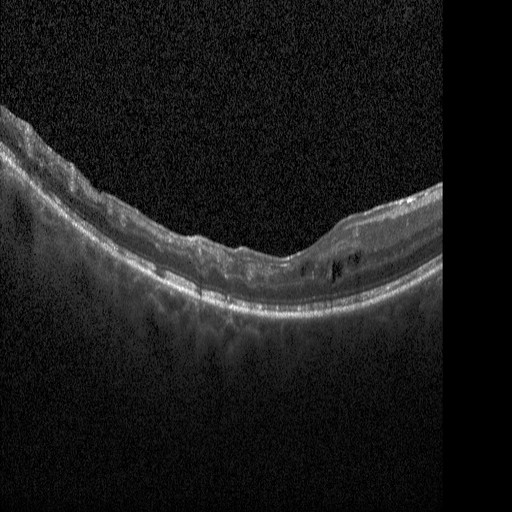

OCT line scan.
Finding: diabetic macular edema (DME).